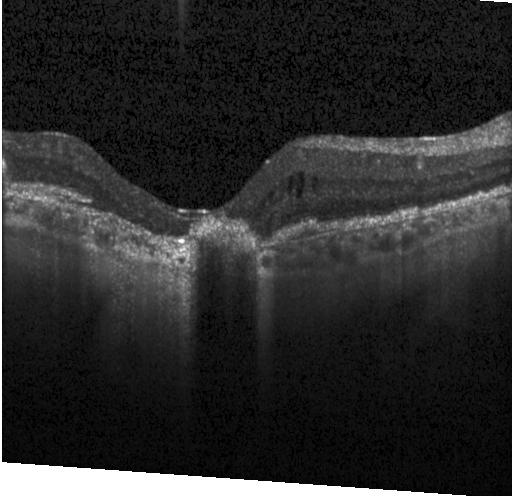

OCT line scan, through the macula, Heidelberg Spectralis.
A choroidal neovascular membrane.